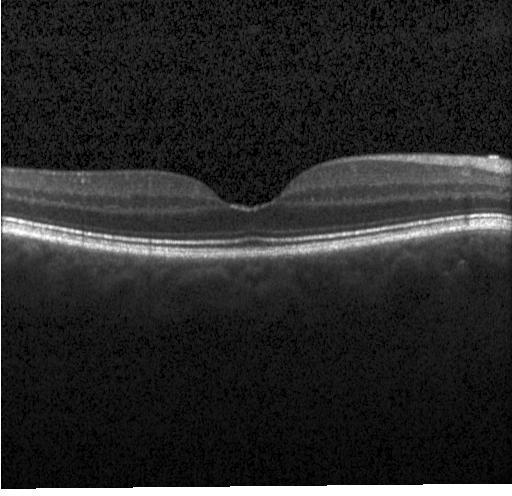

Retinal OCT cross-section — Finding: neither CNV, DME, nor drusen.